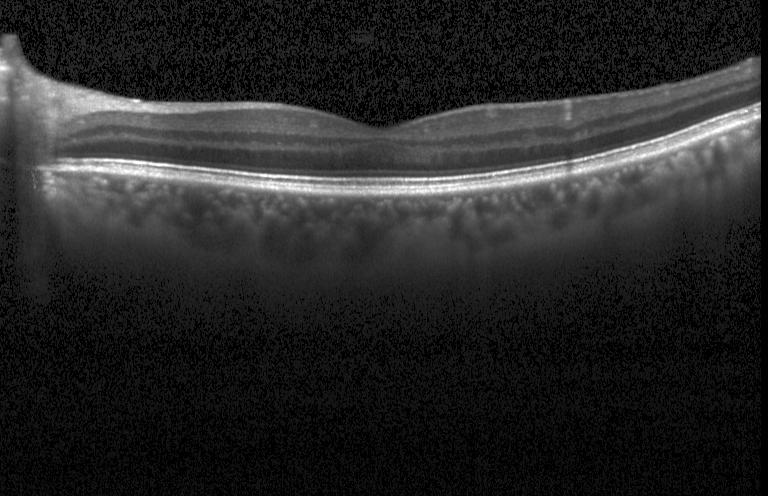

OCT finding: neither choroidal neovascularization, diabetic macular edema, nor drusen.